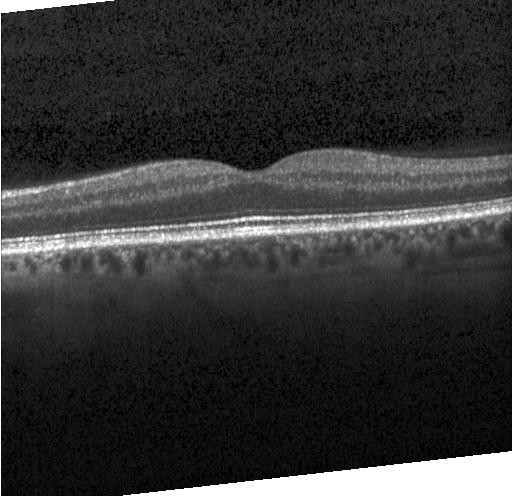 Retinal OCT B-scan
This B-scan demonstrates no choroidal neovascularization, diabetic macular edema, or drusen.